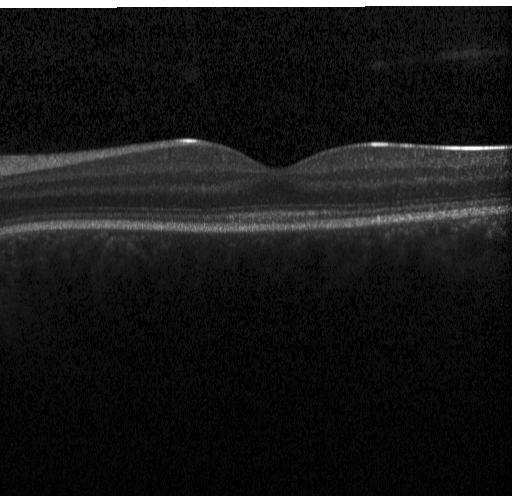
Instrument: Heidelberg Spectralis. Horizontal scan through the fovea. Optical coherence tomography scan. SD-OCT.
Diagnosis: no CNV, DME, or drusen.